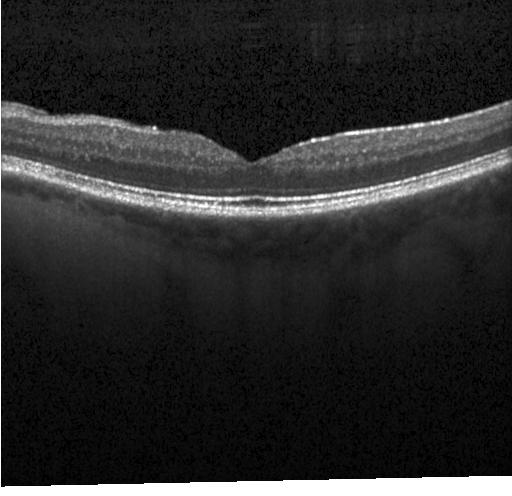 Macular scan · retinal OCT B-scan — OCT finding: no choroidal neovascularization, no diabetic macular edema, and no drusen.